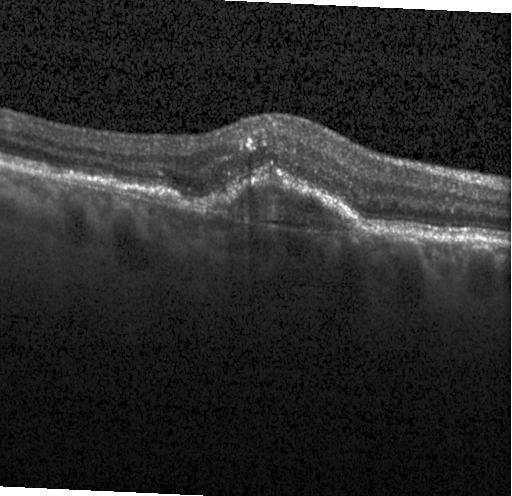 Through the macula; optical coherence tomography B-scan; spectral-domain optical coherence tomography — A choroidal neovascular membrane.